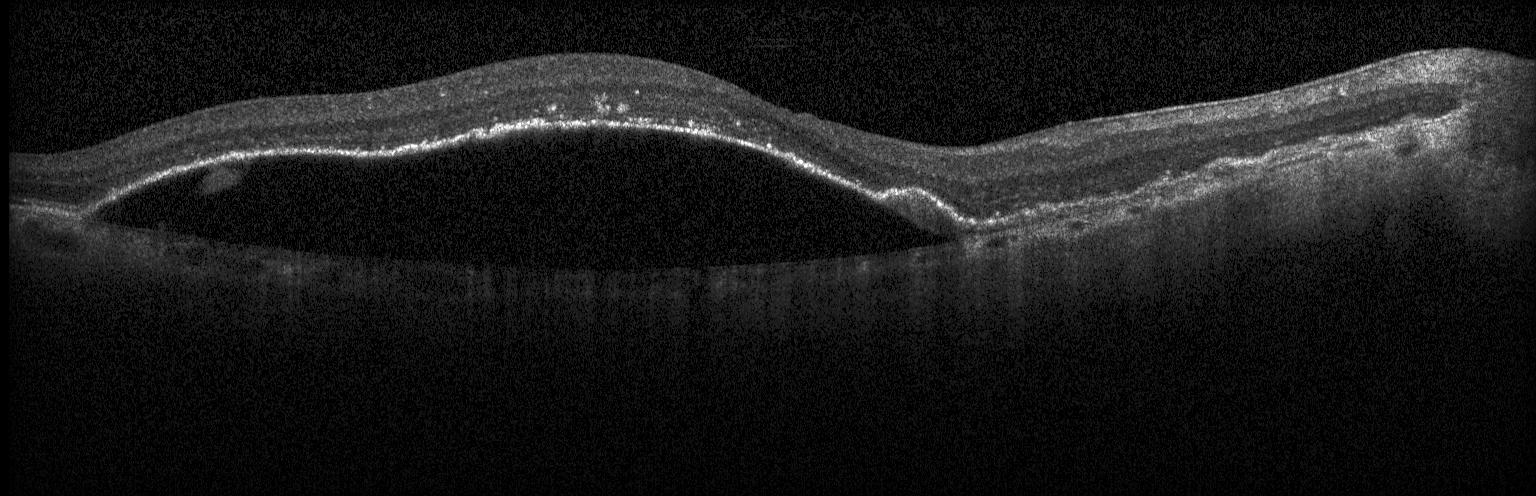 Through the macula, Heidelberg Spectralis OCT system, retinal OCT B-scan, SD-OCT. Finding: a choroidal neovascular membrane.